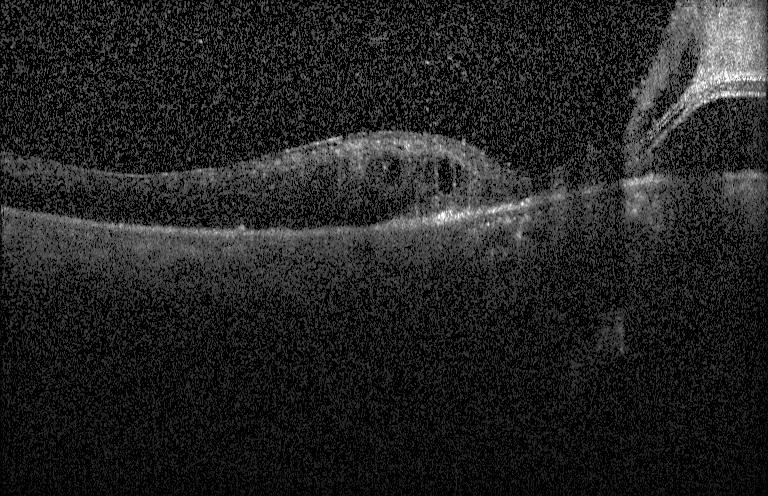 Spectral-domain OCT, retinal OCT B-scan, fovea-centered.
Assessment: diabetic macular edema (DME).